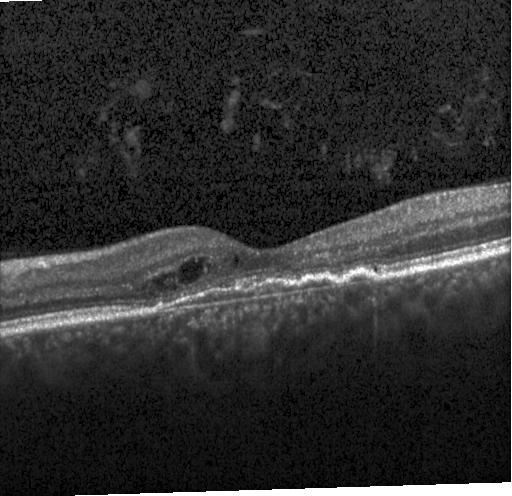 Impression: choroidal neovascularization (CNV).